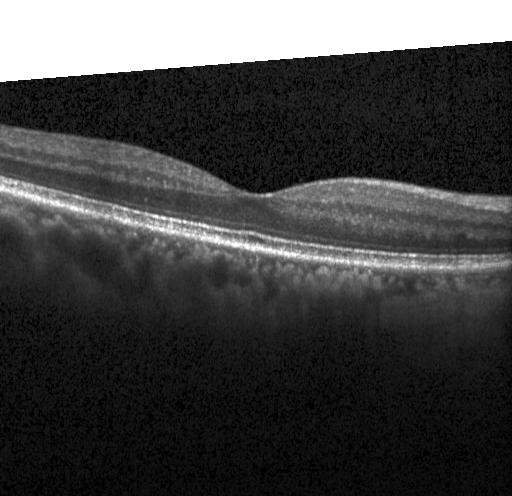

Retinal OCT cross-section
Impression: no evidence of choroidal neovascularization, diabetic macular edema, or drusen.